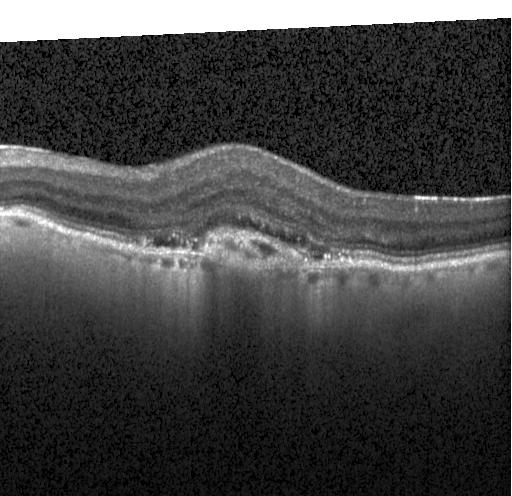

Impression: choroidal neovascularization.